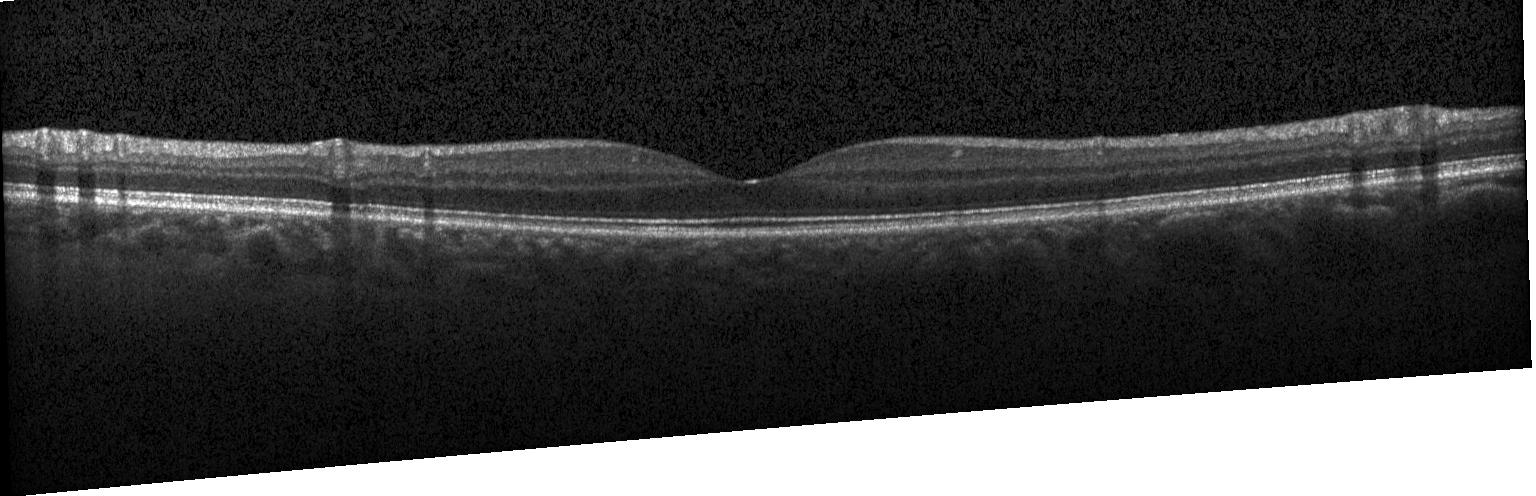 Assessment: no evidence of choroidal neovascularization, diabetic macular edema, or drusen.